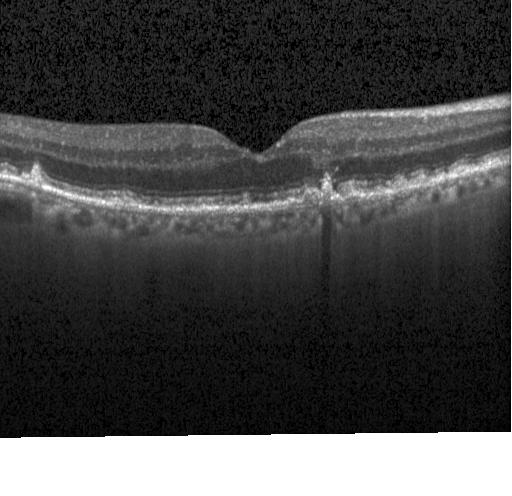

SD-OCT; through the macula; optical coherence tomography B-scan — Diagnosis: sub-RPE drusenoid deposits.